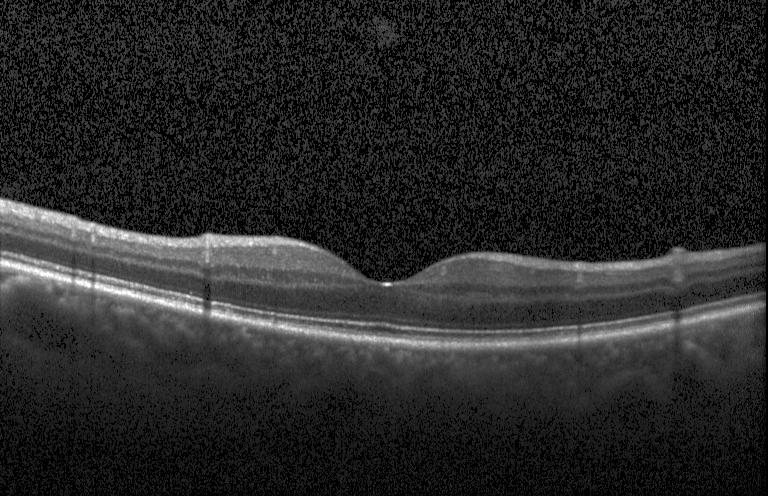 OCT finding: neither choroidal neovascularization, diabetic macular edema, nor drusen.